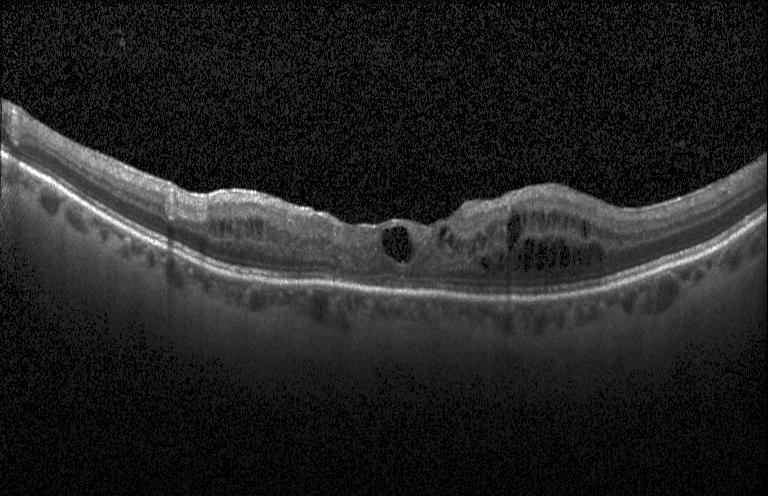
Finding: diabetic macular edema (DME).